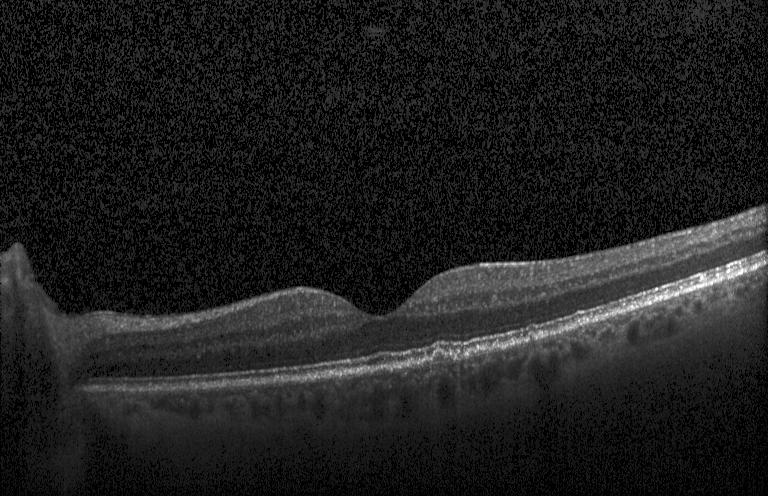
Multiple drusen.